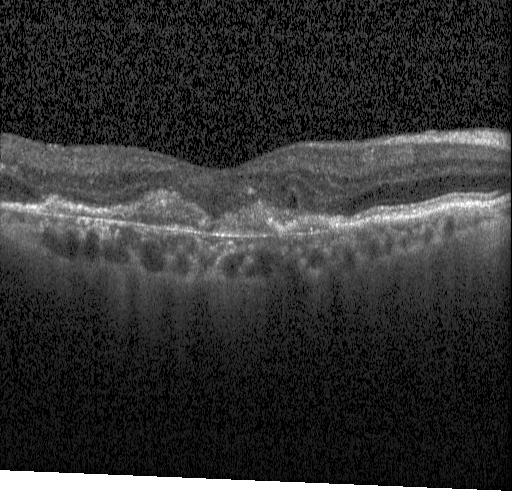
Retinal OCT cross-section showing choroidal neovascularization (CNV).